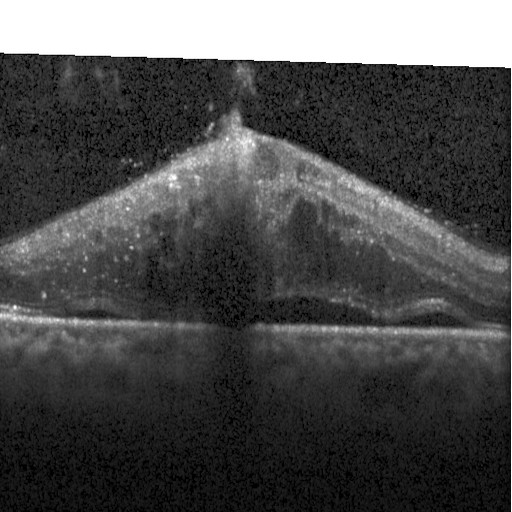

Diagnosis: DME.